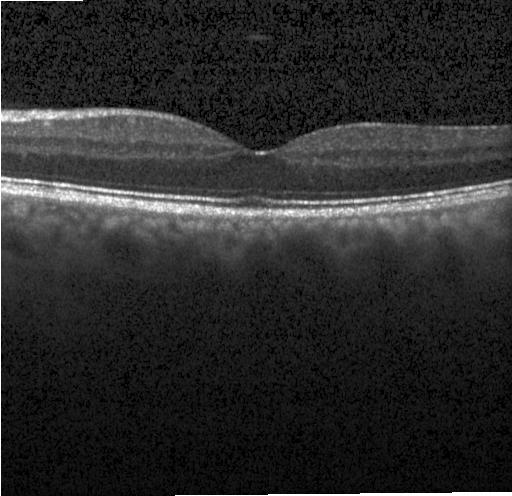 OCT B-scan, fovea-centered, spectral-domain OCT
The scan shows no evidence of choroidal neovascularization, diabetic macular edema, or drusen.